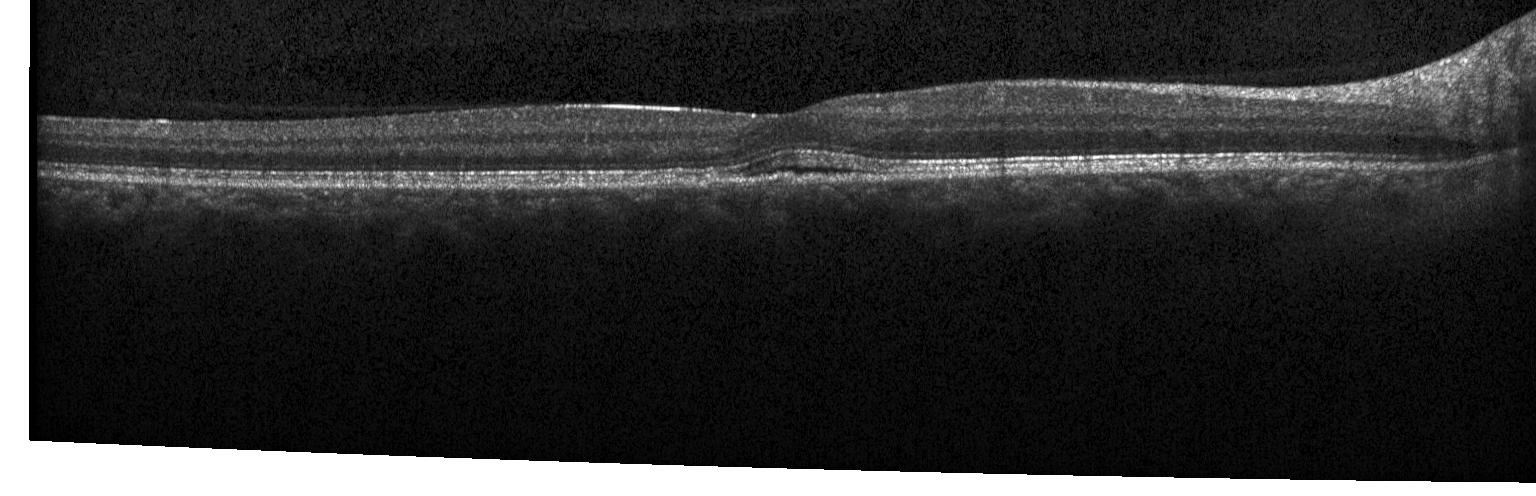 Optical coherence tomography B-scan · centered on the fovea · SD-OCT · Heidelberg Spectralis. The scan shows a choroidal neovascular membrane.